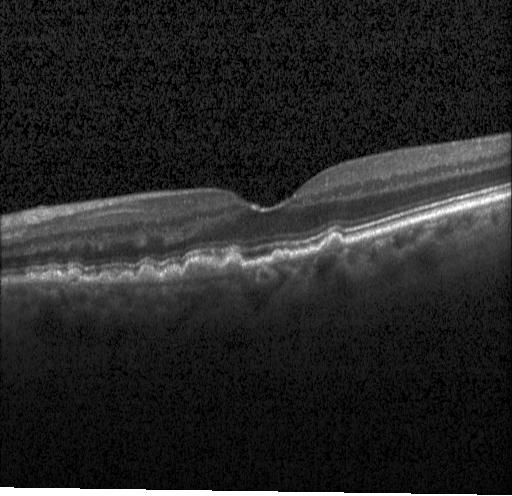 Spectral-domain optical coherence tomography, retinal OCT B-scan
This B-scan demonstrates sub-RPE drusenoid deposits.